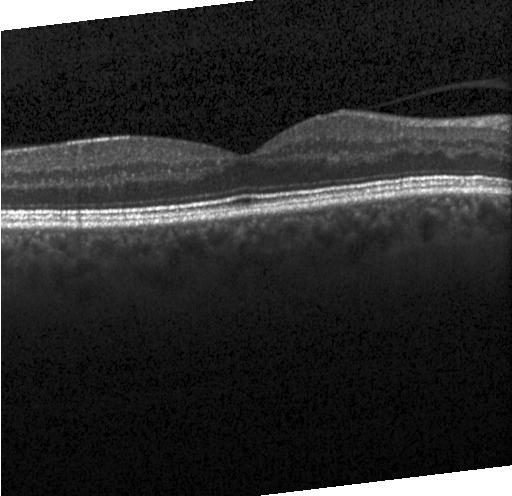 Optical coherence tomography scan, through the macula.
The scan shows no evidence of choroidal neovascularization, diabetic macular edema, or drusen.